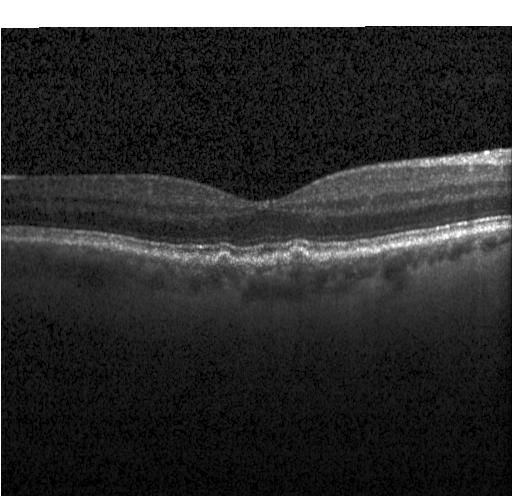 Heidelberg Spectralis · horizontal scan through the fovea · optical coherence tomography B-scan
Finding: multiple drusen.